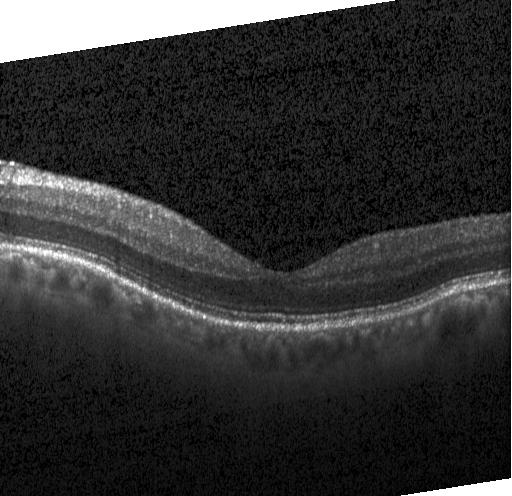

Retinal OCT cross-section.
Impression: no evidence of CNV, DME, or drusen.